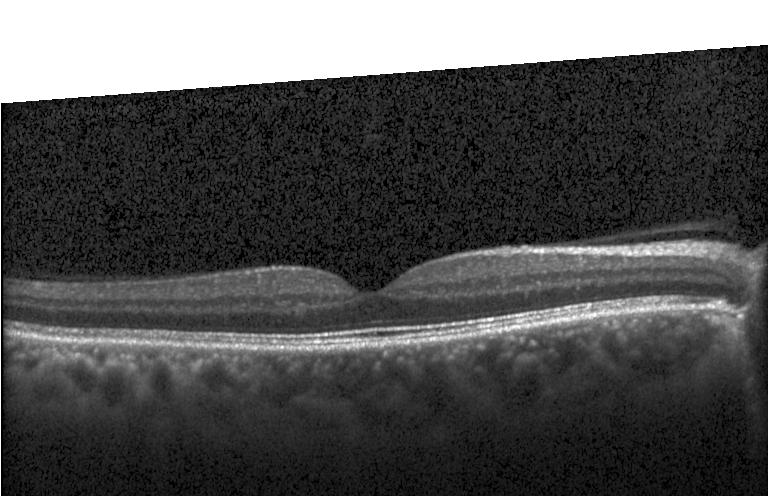
Spectral-domain optical coherence tomography · centered on the fovea · acquired on a Heidelberg Spectralis · optical coherence tomography scan
Diagnosis: neither choroidal neovascularization, diabetic macular edema, nor drusen.